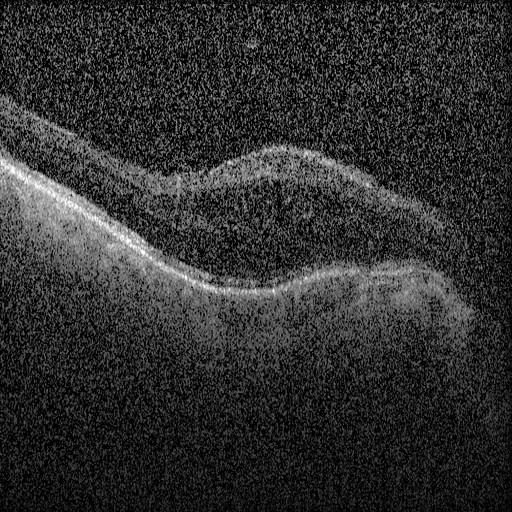 Spectral-domain OCT B-scan: diabetic macular edema (DME).